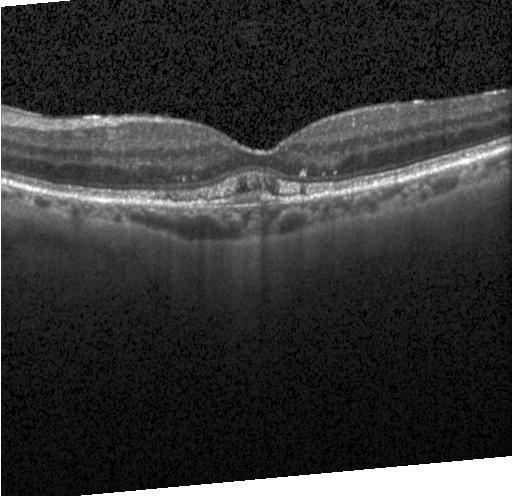 Macular OCT: choroidal neovascularization.